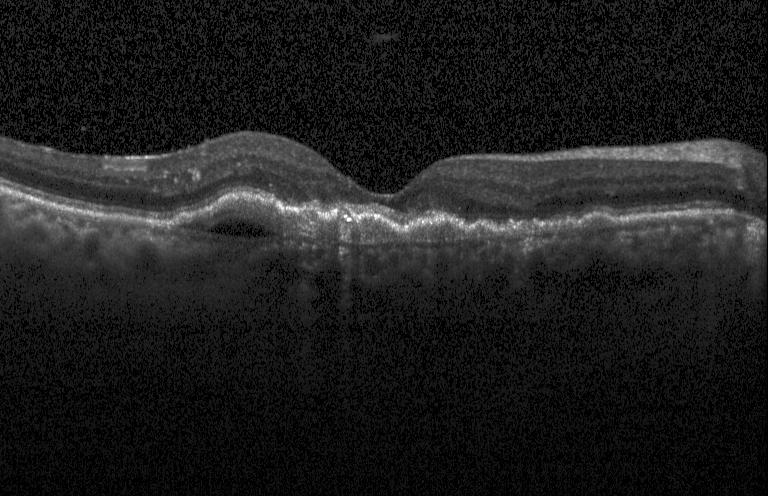

Centered on the fovea. Retinal OCT cross-section. Acquired on a Heidelberg Spectralis
Impression: choroidal neovascularization.